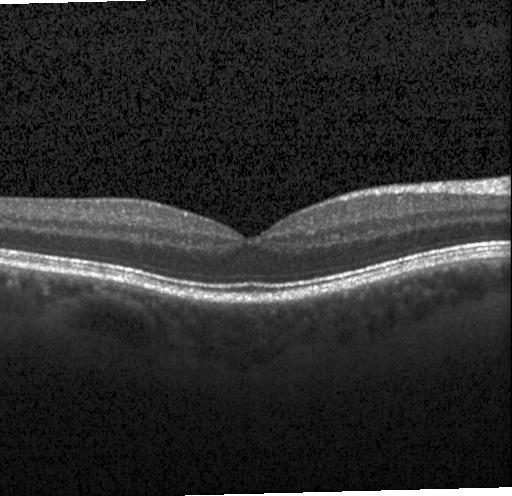 Dx: no choroidal neovascularization, no diabetic macular edema, and no drusen.